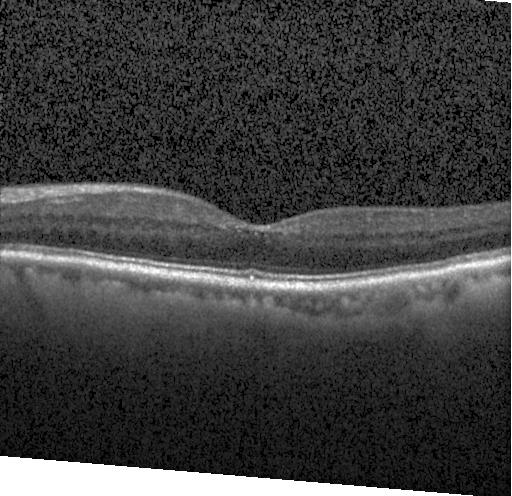
OCT scan showing neither choroidal neovascularization, diabetic macular edema, nor drusen.